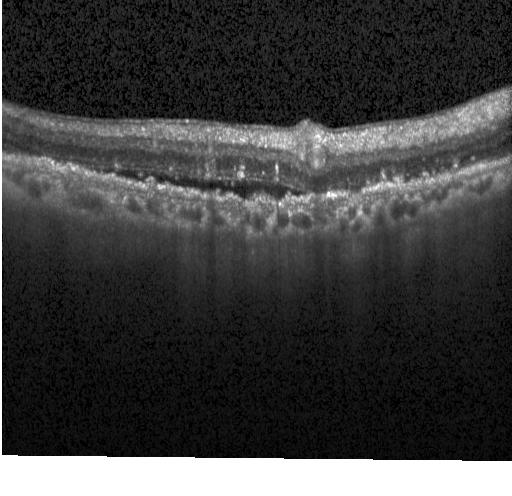
Heidelberg Spectralis OCT system; spectral-domain optical coherence tomography; optical coherence tomography scan — Dx: choroidal neovascularization.